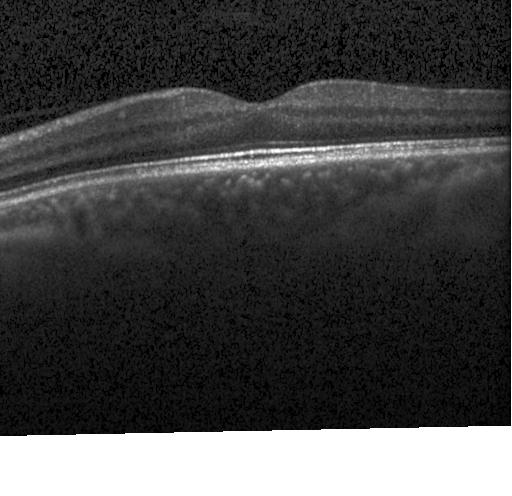

Retinal OCT cross-section. Finding: no choroidal neovascularization, diabetic macular edema, or drusen.